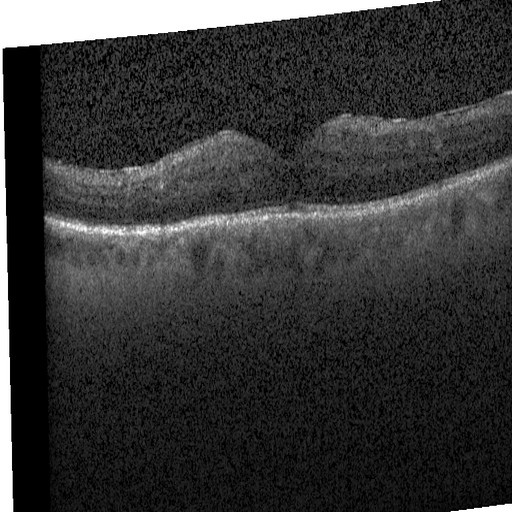 Macular OCT: diabetic macular edema.